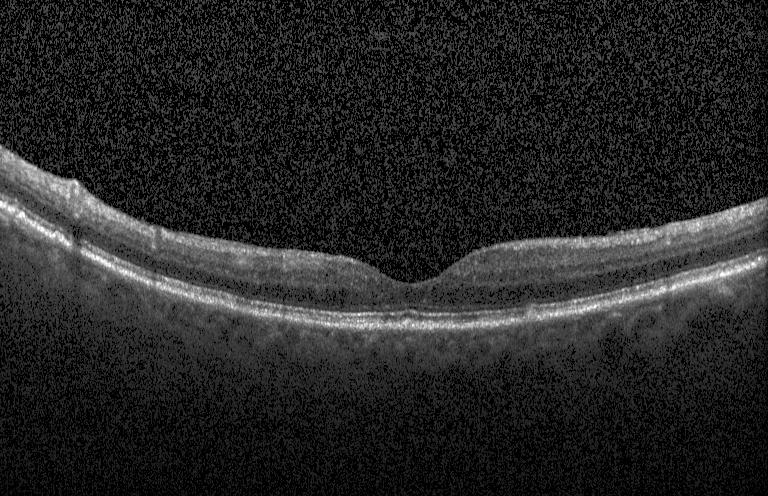 Macular scan; retinal OCT B-scan; spectral-domain optical coherence tomography
Impression: no evidence of choroidal neovascularization, diabetic macular edema, or drusen.